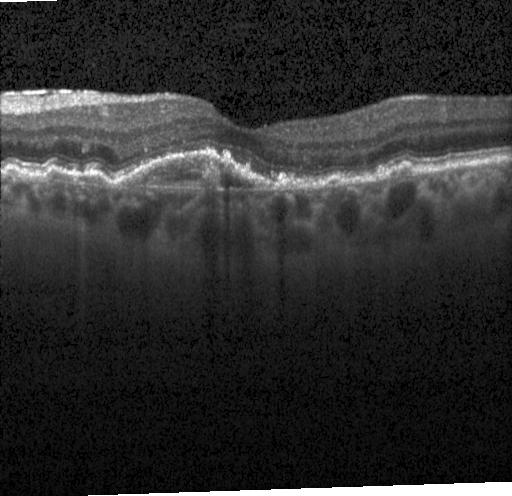

OCT B-scan showing a choroidal neovascular membrane.